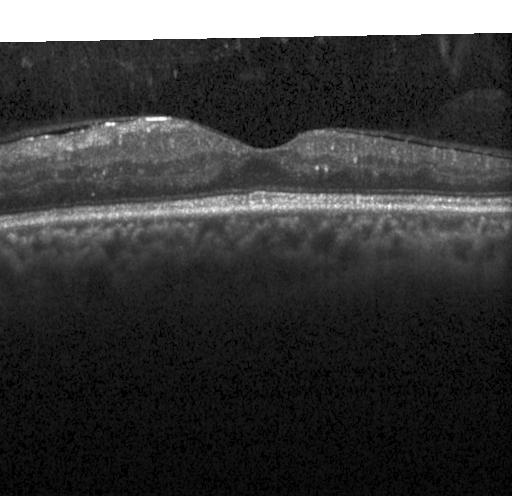

Retinal OCT cross-section showing diabetic macular edema.